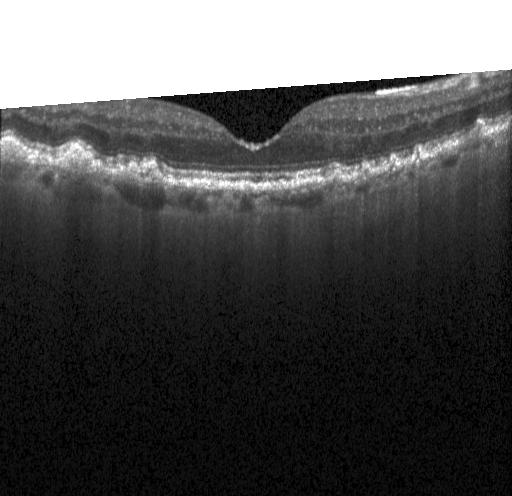

Optical coherence tomography B-scan · spectral-domain OCT — Dx: drusen.